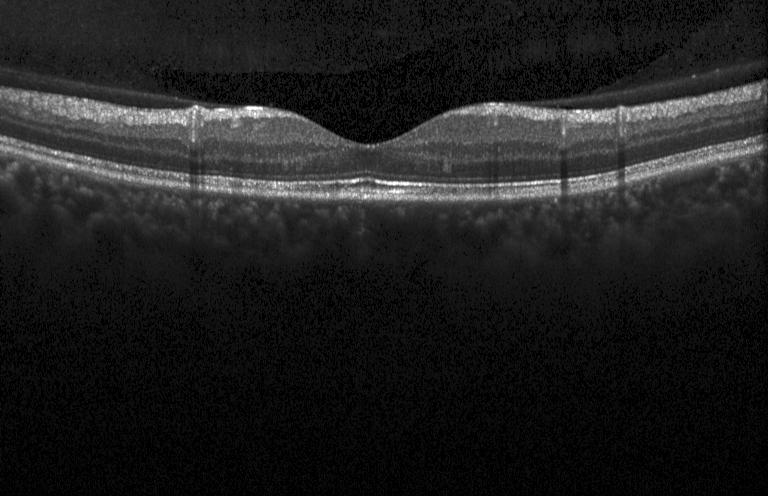 Retinal OCT cross-section — Impression: no evidence of CNV, DME, or drusen.